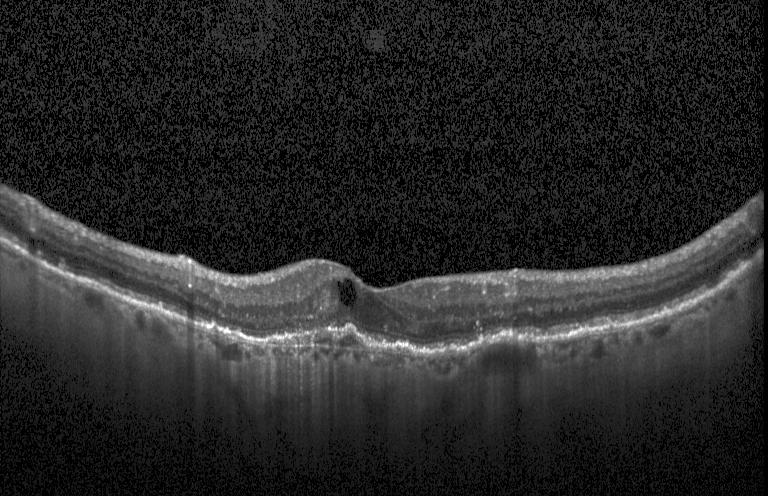 OCT line scan · Heidelberg Spectralis OCT system · fovea-centered — The scan shows a choroidal neovascular membrane.